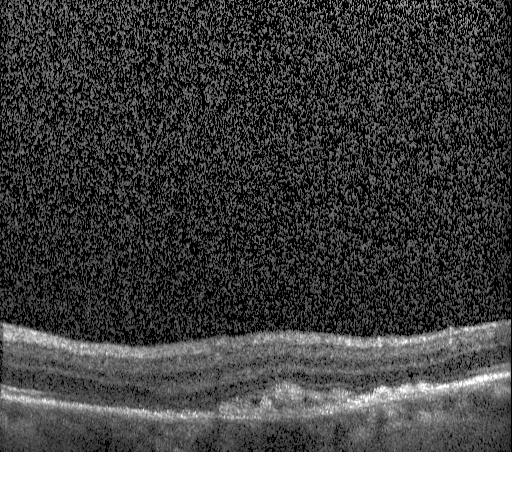

Retinal OCT cross-section · spectral-domain OCT · Heidelberg Spectralis · centered on the fovea. The scan shows a choroidal neovascular membrane.